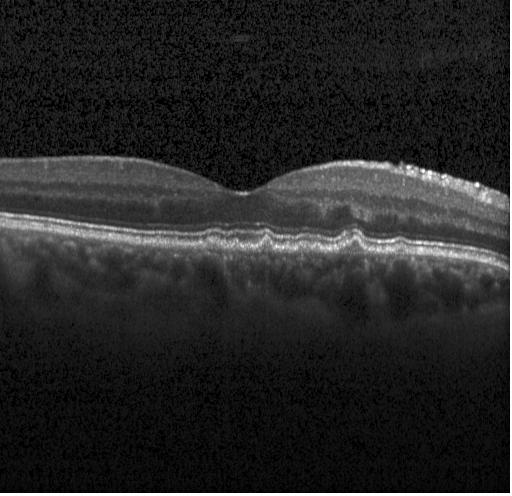 Optical coherence tomography B-scan; macular scan; spectral-domain optical coherence tomography
Macular OCT: drusen.